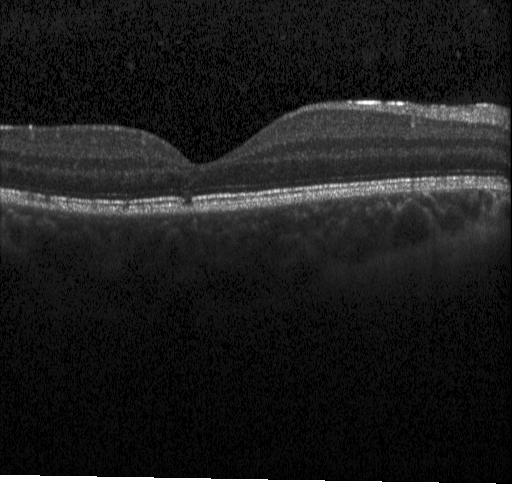
Through the macula. Acquired on a Heidelberg Spectralis. Retinal OCT cross-section. Assessment: neither choroidal neovascularization, diabetic macular edema, nor drusen.